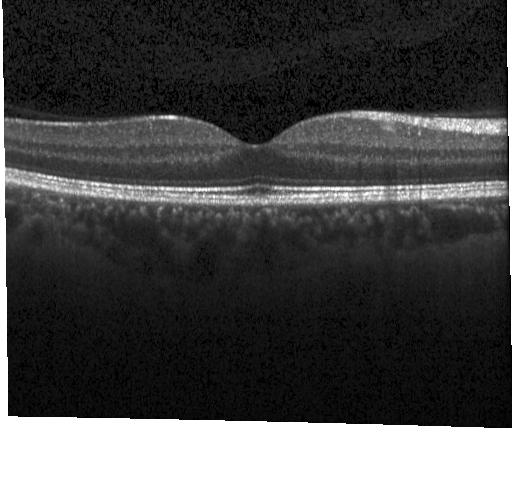 Optical coherence tomography scan · Heidelberg Spectralis.
Macular OCT: no choroidal neovascularization, no diabetic macular edema, and no drusen.